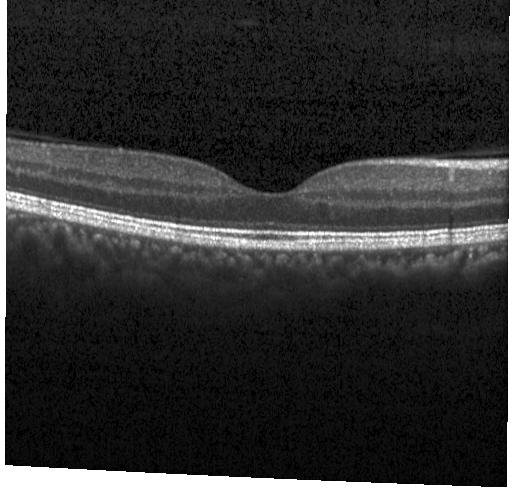

OCT scan showing no choroidal neovascularization, no diabetic macular edema, and no drusen.